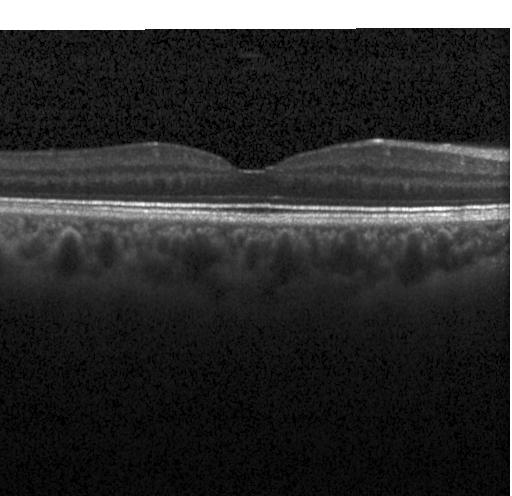
OCT B-scan showing no evidence of CNV, DME, or drusen.